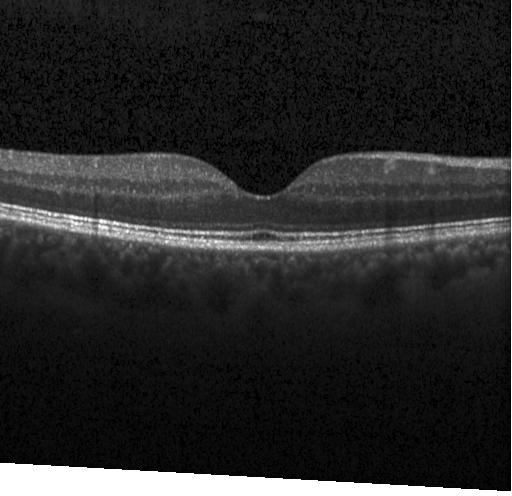 Retinal OCT cross-section · spectral-domain OCT — Diagnosis: neither CNV, DME, nor drusen.